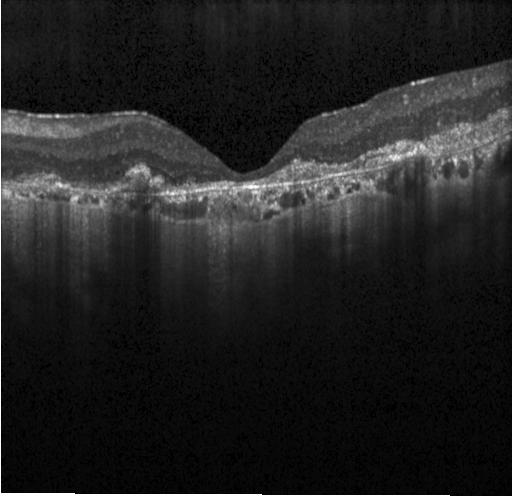 Finding: choroidal neovascularization.